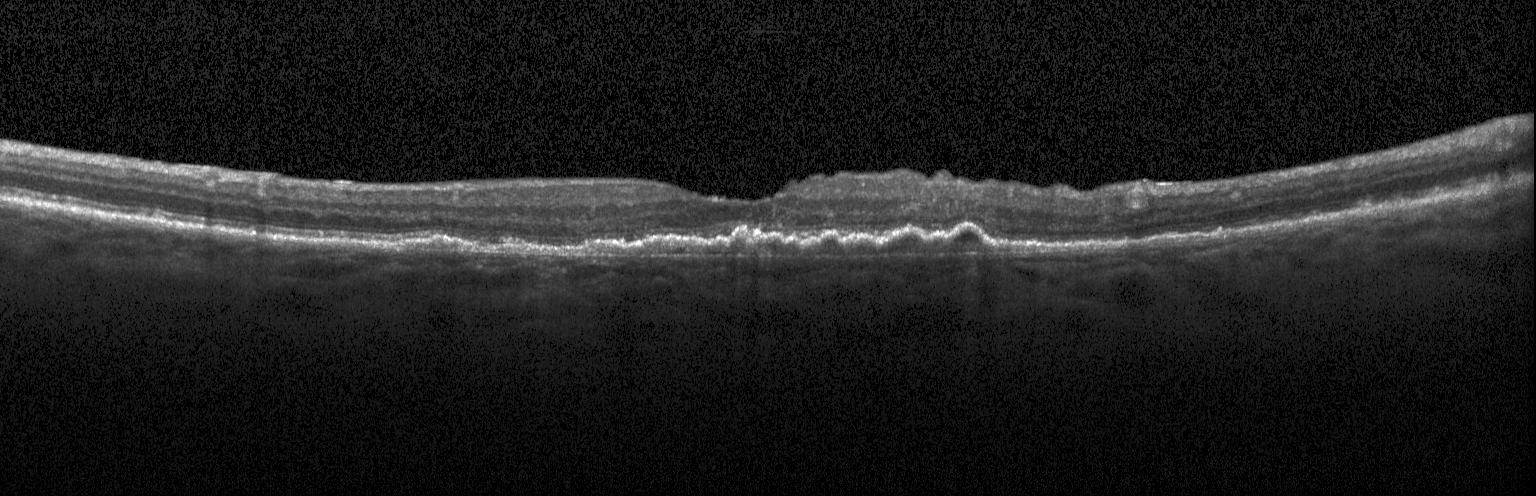 Acquired on a Heidelberg Spectralis, SD-OCT, through the macula, retinal OCT cross-section.
Assessment: a choroidal neovascular membrane.